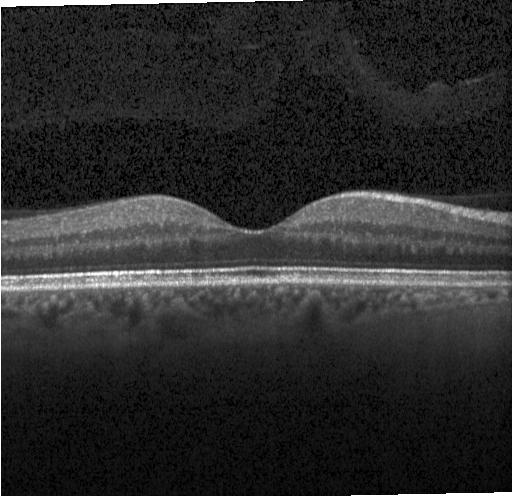
Macular scan; optical coherence tomography scan.
OCT finding: no choroidal neovascularization, no diabetic macular edema, and no drusen.